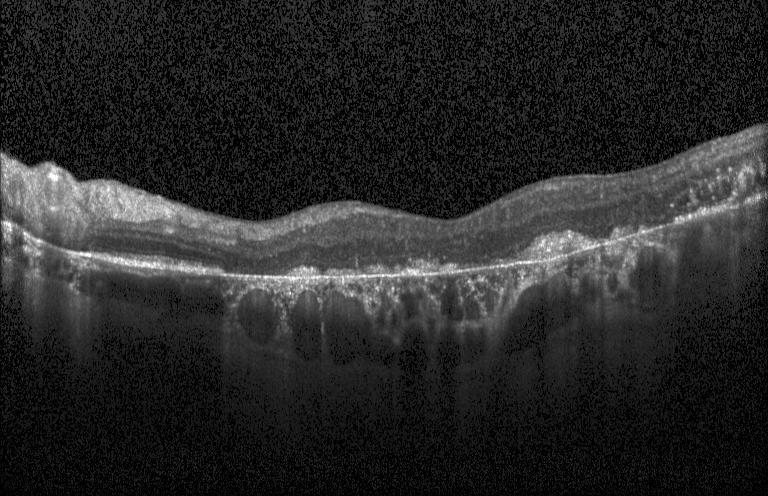

Optical coherence tomography scan, centered on the fovea. Choroidal neovascularization (CNV).